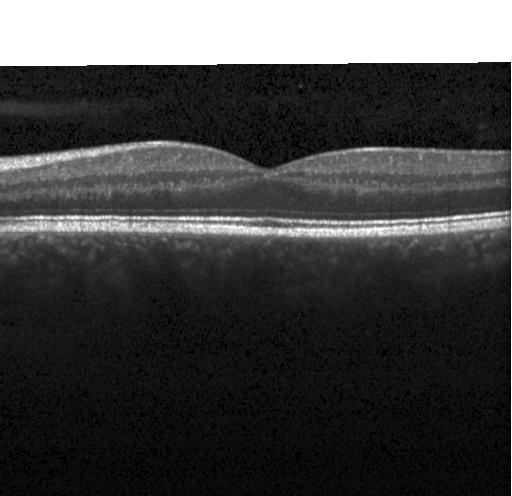

Assessment: no choroidal neovascularization, diabetic macular edema, or drusen.